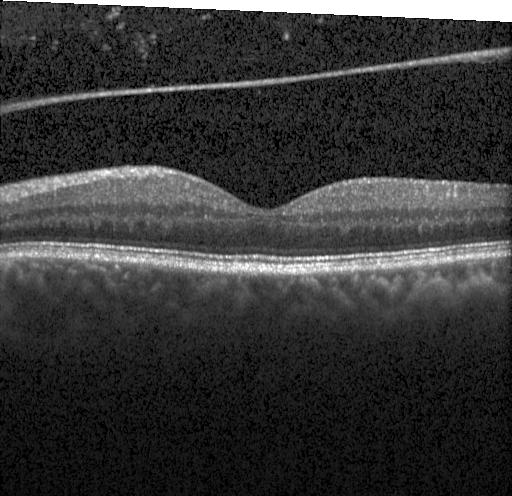

OCT B-scan showing no choroidal neovascularization, diabetic macular edema, or drusen.